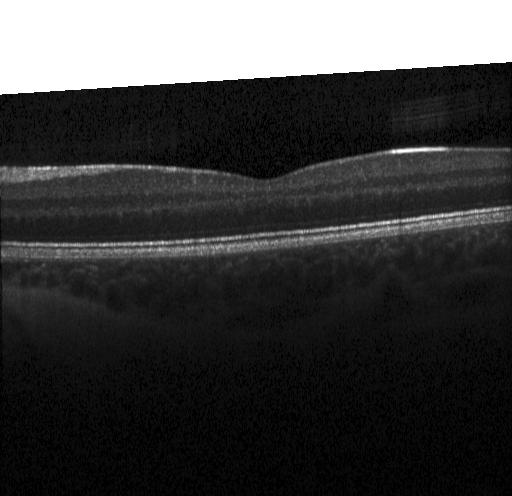
Macular OCT: no choroidal neovascularization, diabetic macular edema, or drusen.